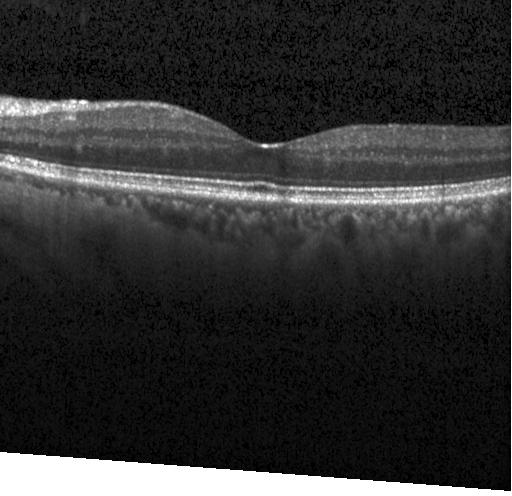 Retinal OCT cross-section showing no evidence of CNV, DME, or drusen.